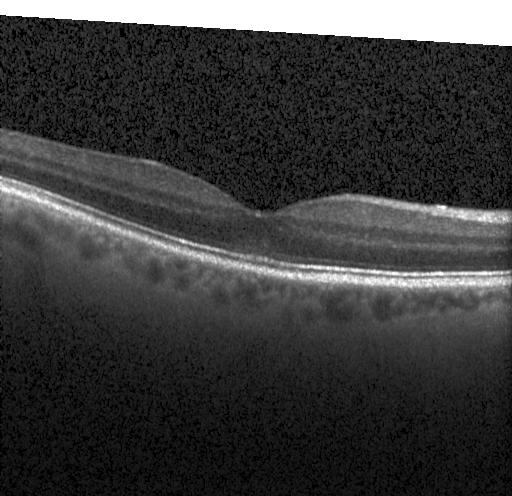
Retinal OCT cross-section showing neither choroidal neovascularization, diabetic macular edema, nor drusen.